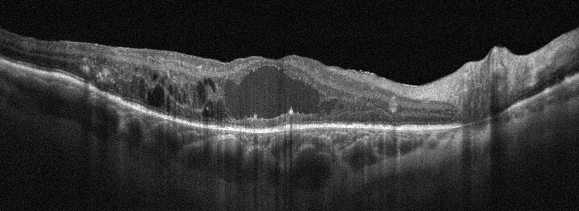
OCT B-scan; OD; macular scan; Optovue Avanti RTVue XR.
Diabetic macular edema (DME).